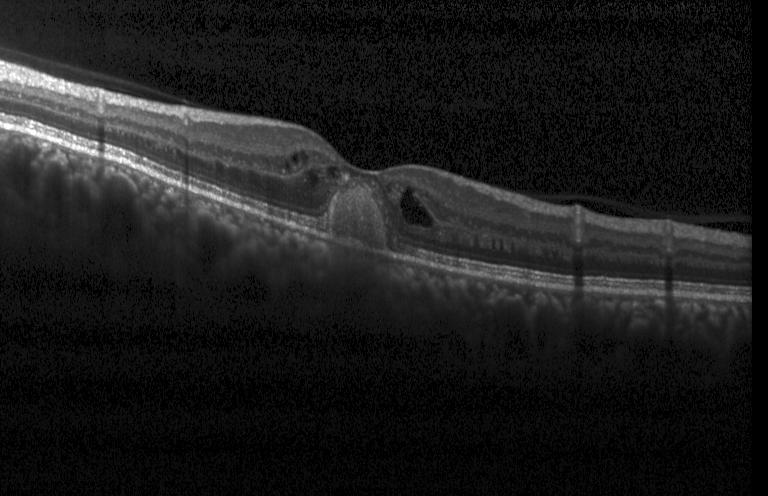 Heidelberg Spectralis. Retinal OCT B-scan
Impression: a choroidal neovascular membrane.